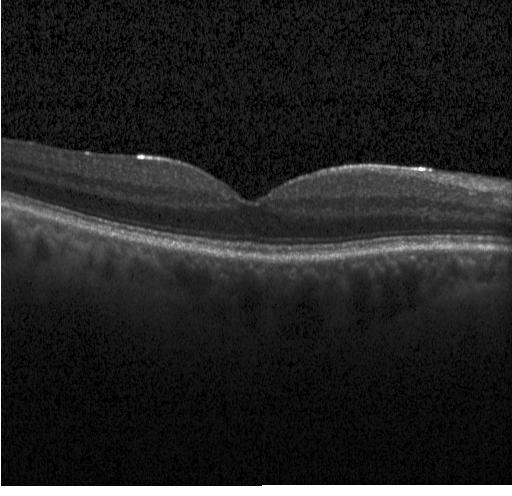

Acquired on a Heidelberg Spectralis, spectral-domain OCT, OCT B-scan. Finding: neither CNV, DME, nor drusen.